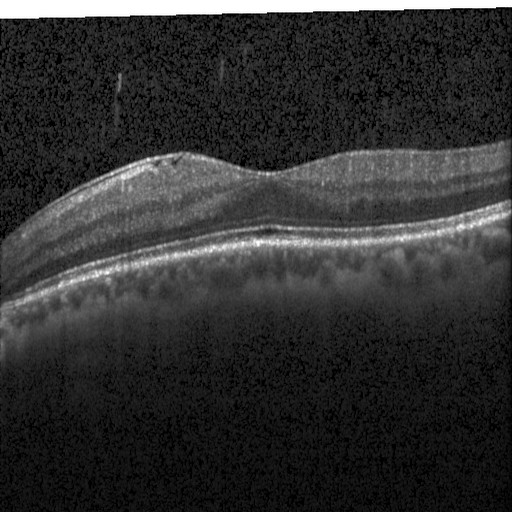

Macular scan, Heidelberg Spectralis OCT system, spectral-domain OCT, optical coherence tomography scan. Diabetic macular edema (DME).